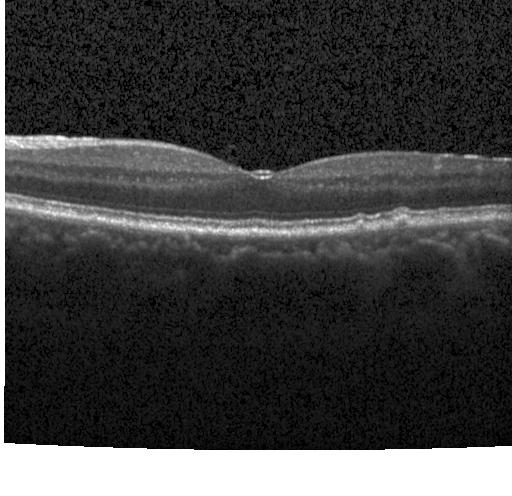
Spectral-domain optical coherence tomography · acquired on a Heidelberg Spectralis · retinal OCT B-scan · fovea-centered — This B-scan demonstrates drusen.